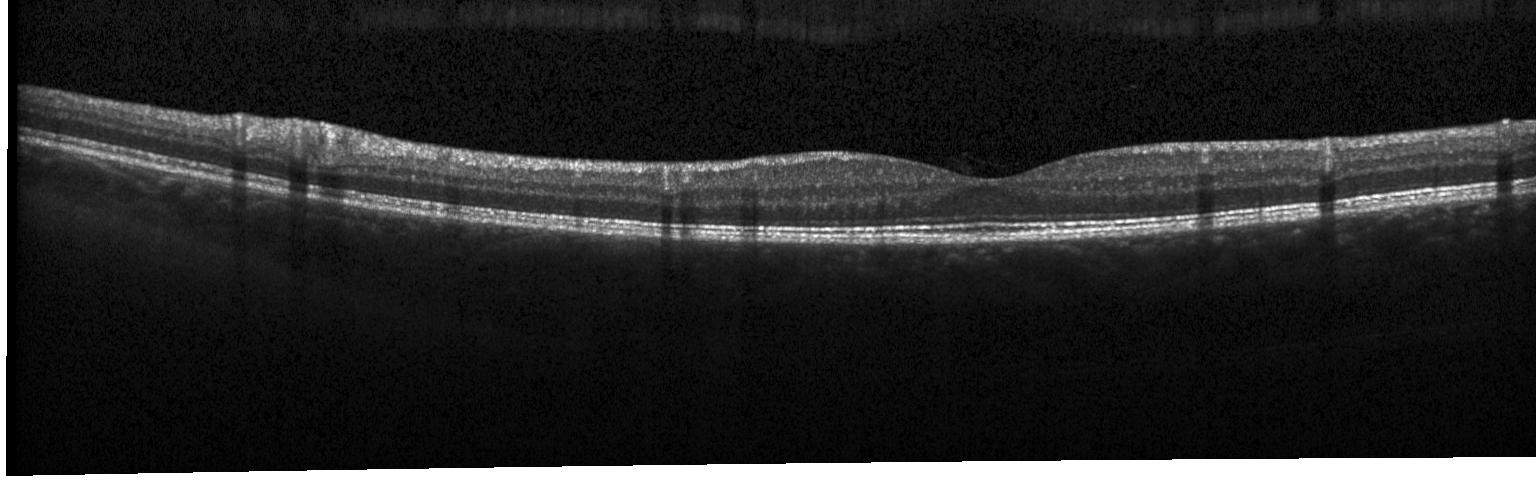
Dx: no choroidal neovascularization, diabetic macular edema, or drusen.